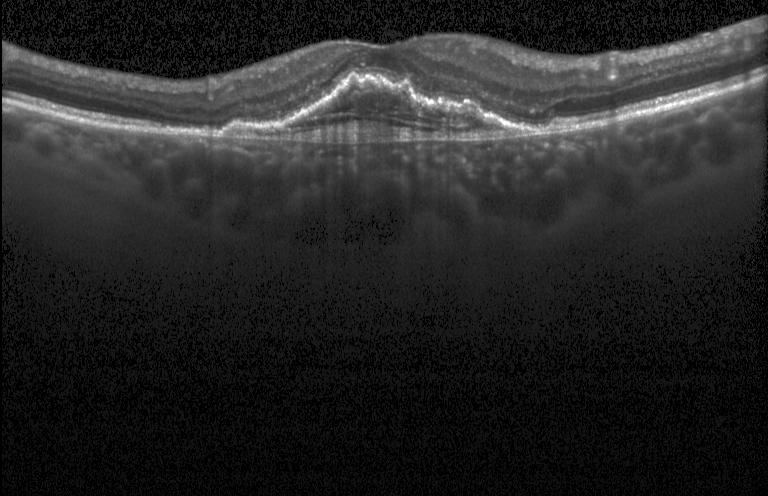
This B-scan demonstrates a choroidal neovascular membrane.